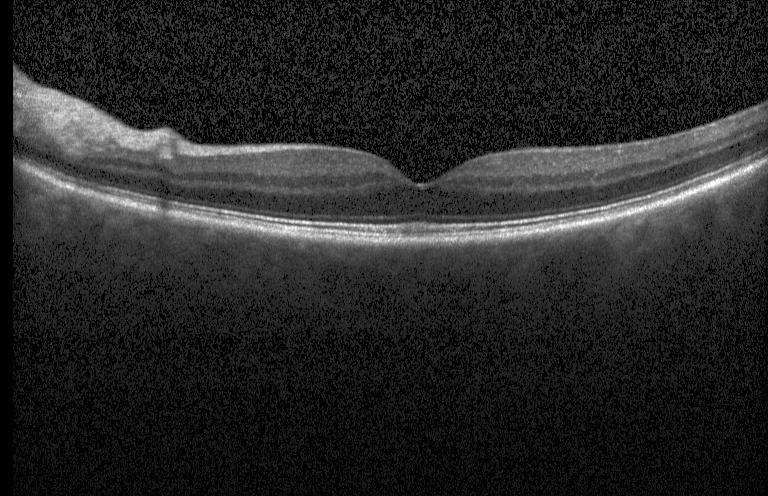 OCT scan showing neither choroidal neovascularization, diabetic macular edema, nor drusen.